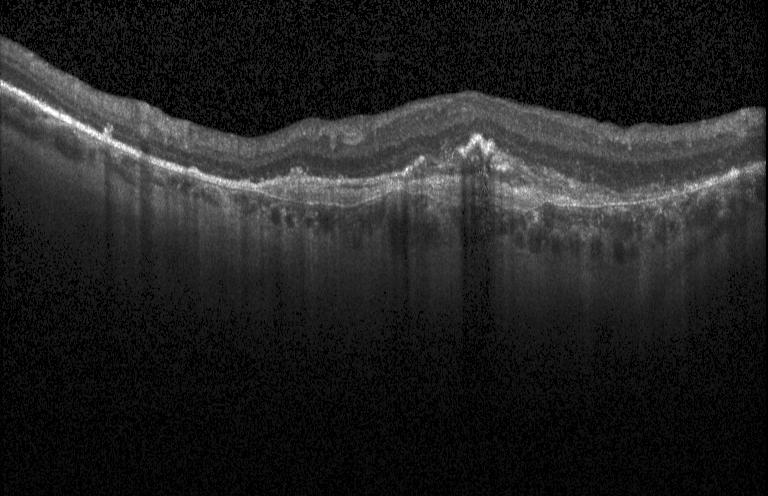
This B-scan demonstrates choroidal neovascularization (CNV).